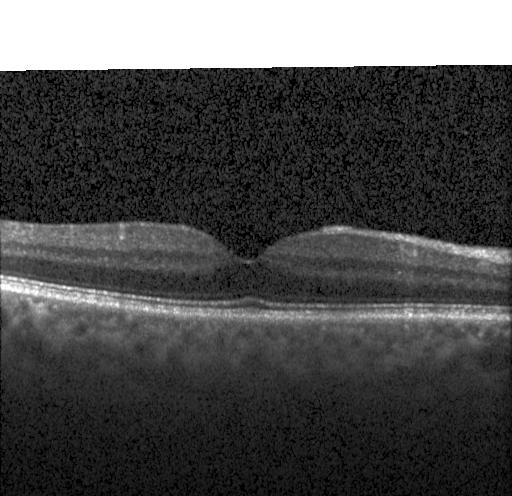

Macular OCT: no choroidal neovascularization, diabetic macular edema, or drusen.